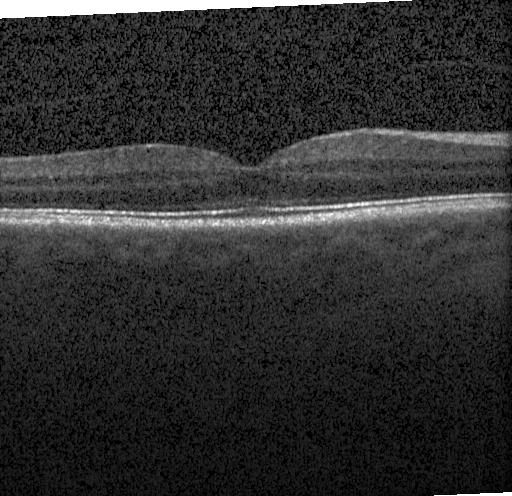
No choroidal neovascularization, diabetic macular edema, or drusen.